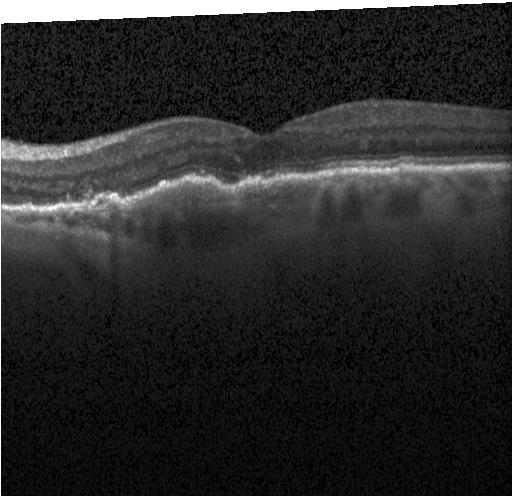
Optical coherence tomography B-scan, fovea-centered. Impression: a choroidal neovascular membrane.